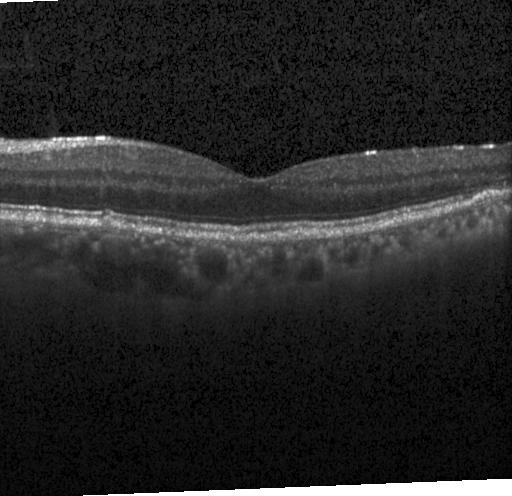 Heidelberg Spectralis · OCT line scan · centered on the fovea — Impression: drusen.